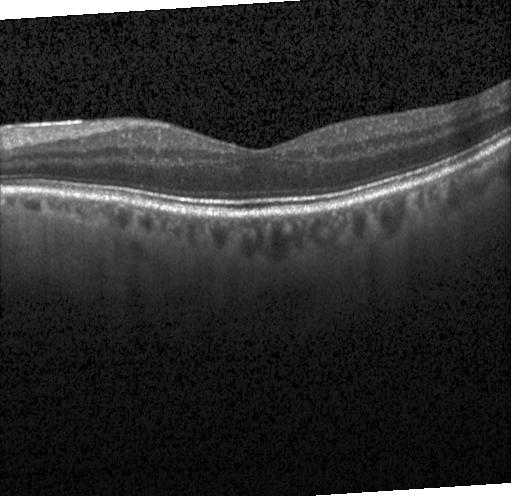 Heidelberg Spectralis · horizontal scan through the fovea · optical coherence tomography B-scan
This B-scan demonstrates no evidence of CNV, DME, or drusen.